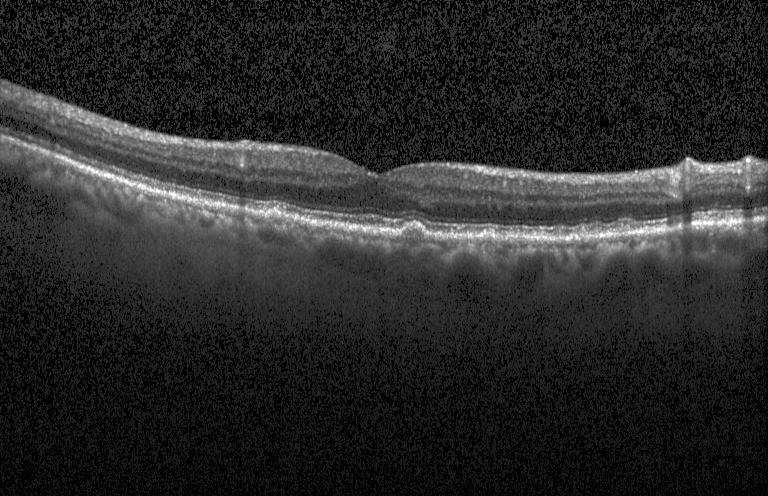 Retinal OCT cross-section · SD-OCT · fovea-centered. OCT finding: sub-RPE drusenoid deposits.